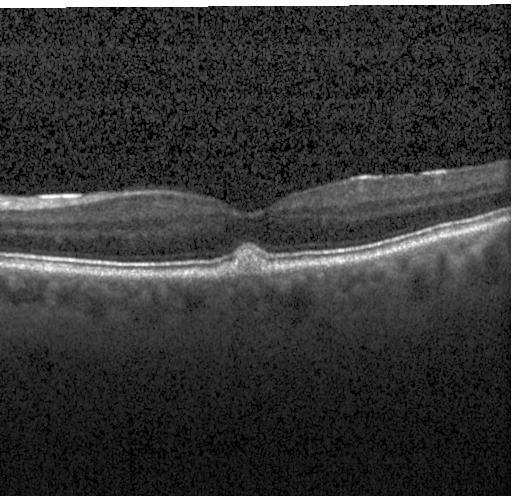 OCT B-scan showing sub-RPE drusenoid deposits.